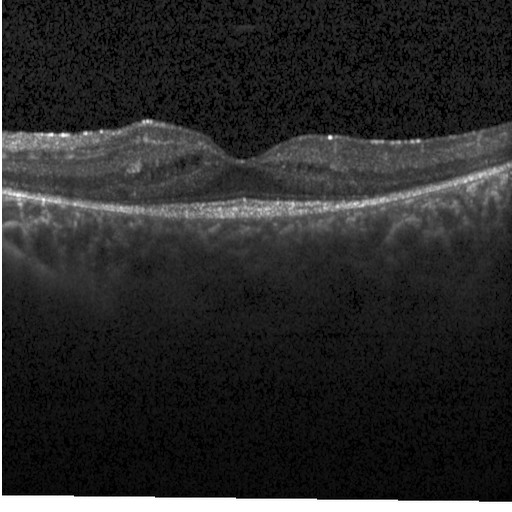
Optical coherence tomography scan
Finding: diabetic macular edema (DME).